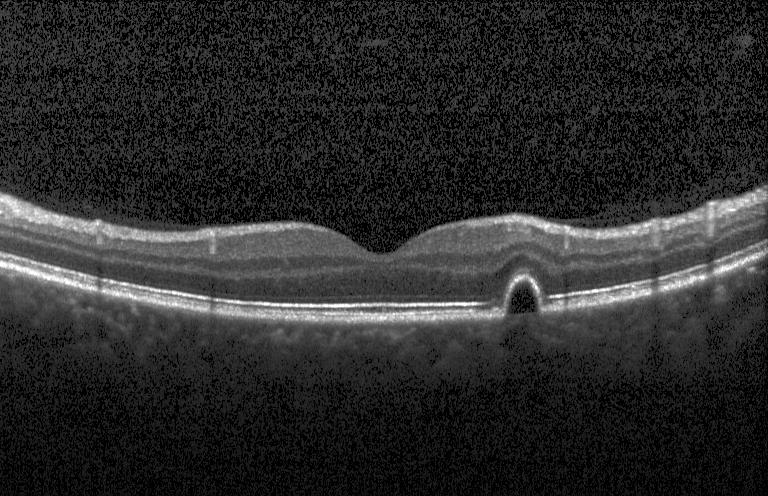

Finding: choroidal neovascularization (CNV).